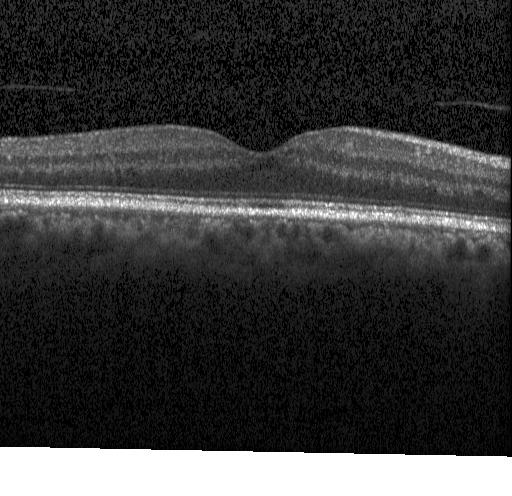
OCT line scan · spectral-domain optical coherence tomography. Impression: no choroidal neovascularization, diabetic macular edema, or drusen.